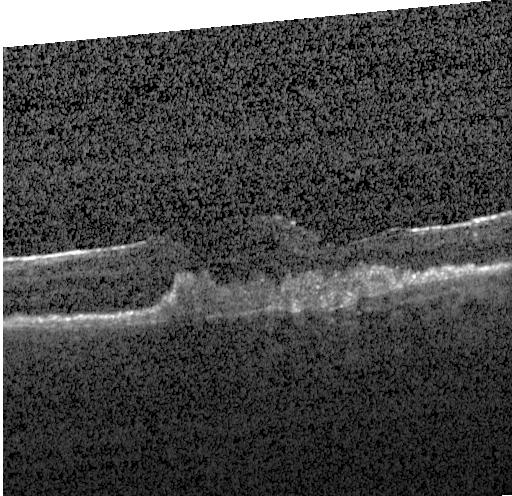

Finding: a choroidal neovascular membrane.